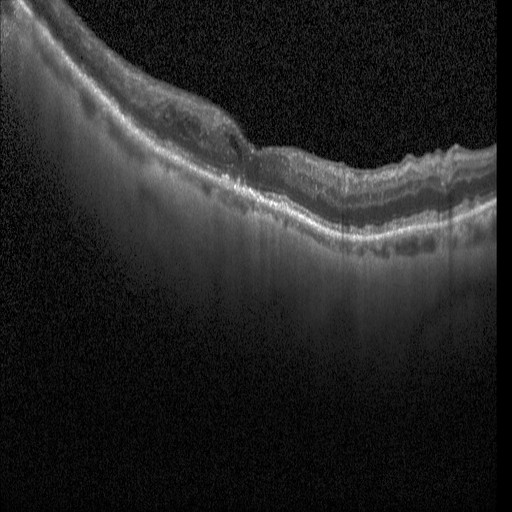
Optical coherence tomography scan; horizontal scan through the fovea; spectral-domain OCT.
Diagnosis: diabetic macular edema.